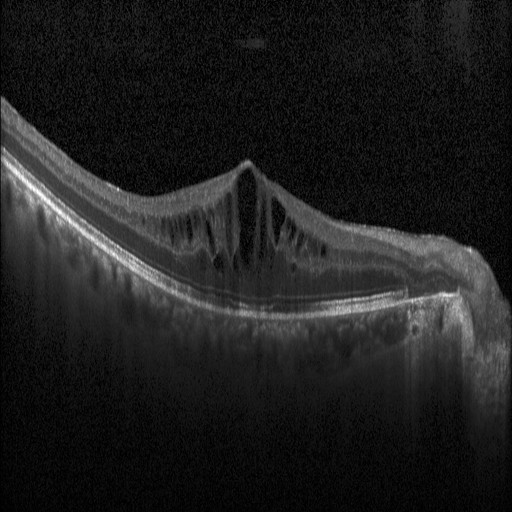

OCT B-scan. Spectral-domain OCT. Heidelberg Spectralis. Macular scan — The scan shows diabetic macular edema.